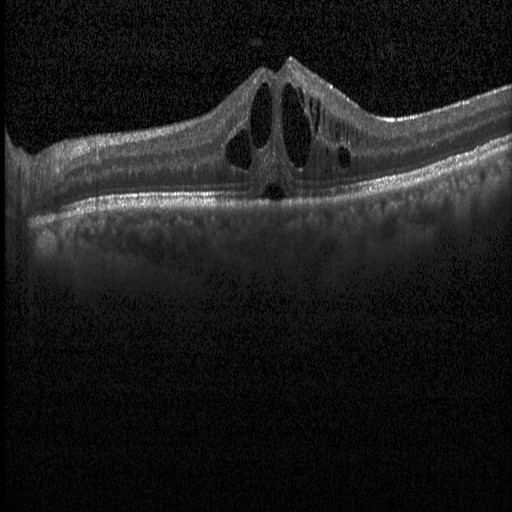
Diabetic macular edema (DME).